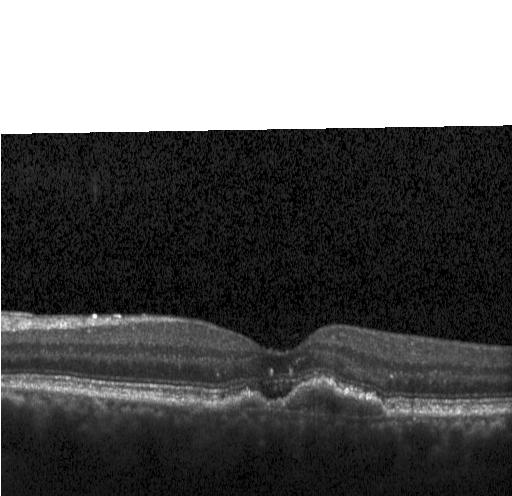 Spectral-domain optical coherence tomography · fovea-centered · Heidelberg Spectralis · OCT B-scan. Finding: a choroidal neovascular membrane.